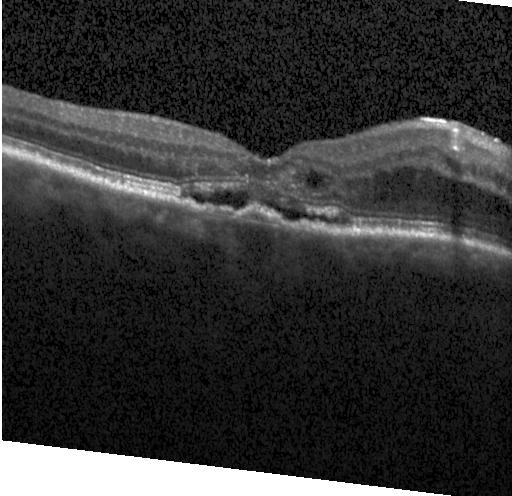

OCT finding: choroidal neovascularization.